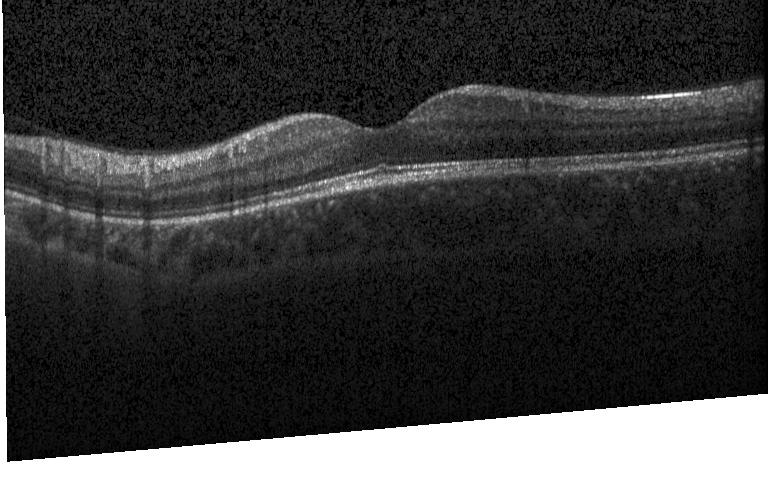
No CNV, no DME, and no drusen.